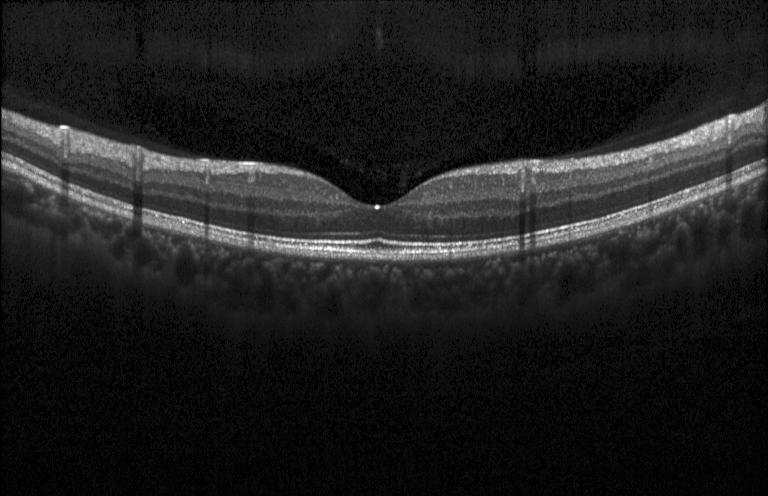

Impression: no evidence of choroidal neovascularization, diabetic macular edema, or drusen.